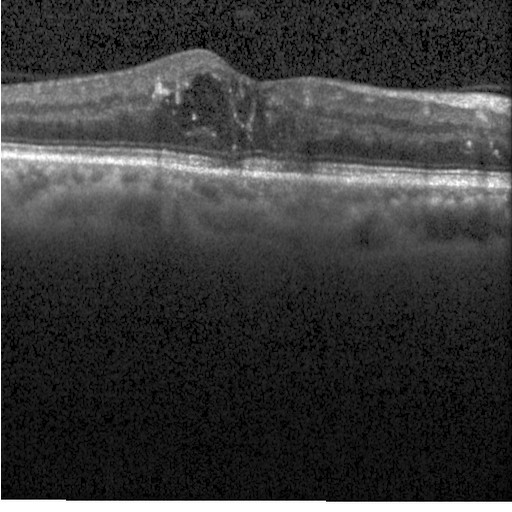 Retinal OCT B-scan; spectral-domain OCT; Heidelberg Spectralis. OCT finding: diabetic macular edema.